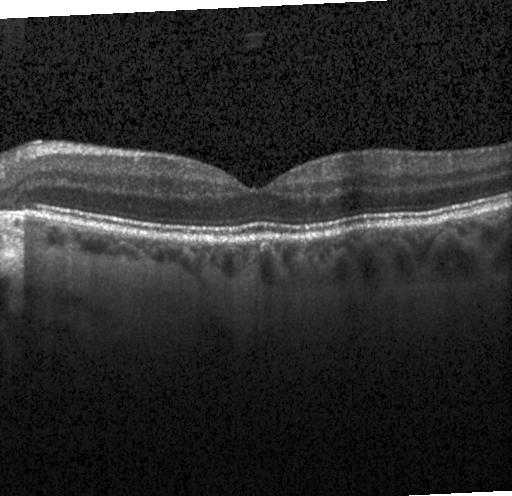

OCT finding: no choroidal neovascularization, no diabetic macular edema, and no drusen.